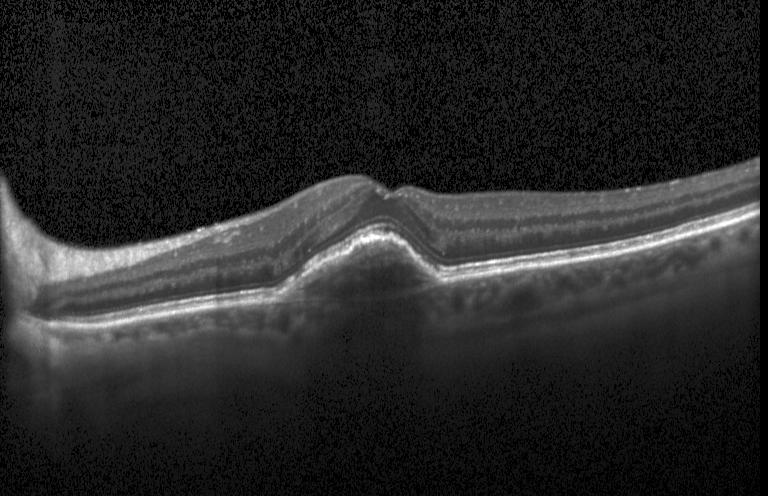
Finding: choroidal neovascularization (CNV).